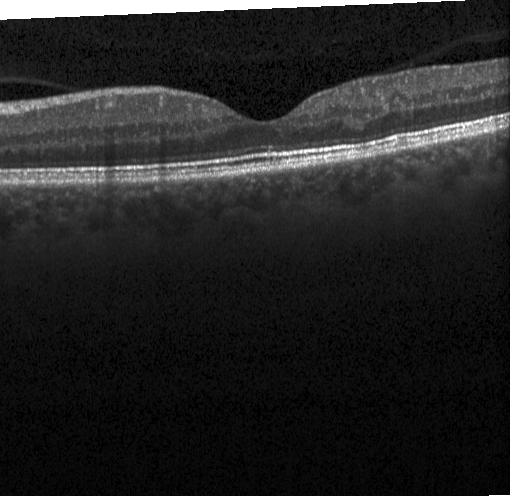
Retinal OCT cross-section. Spectral-domain optical coherence tomography. Centered on the fovea — Finding: no choroidal neovascularization, no diabetic macular edema, and no drusen.